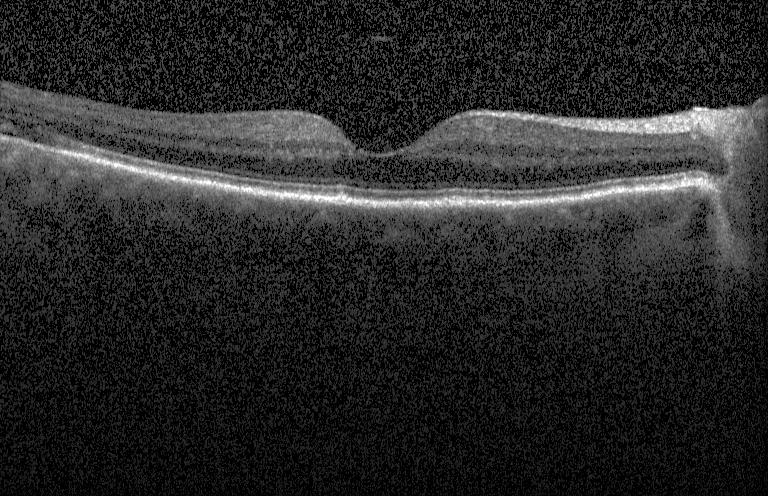

Macular OCT: no CNV, no DME, and no drusen.